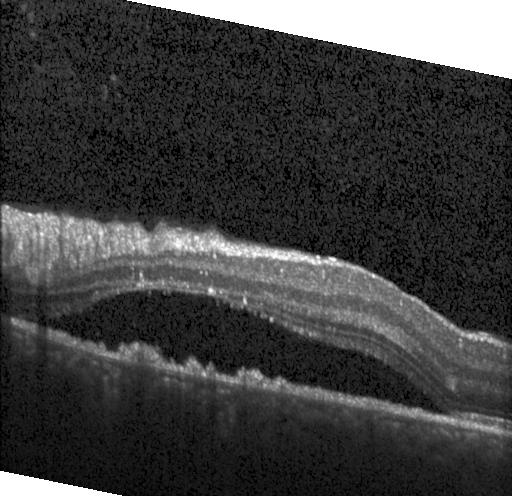

Optical coherence tomography B-scan
Finding: a choroidal neovascular membrane.